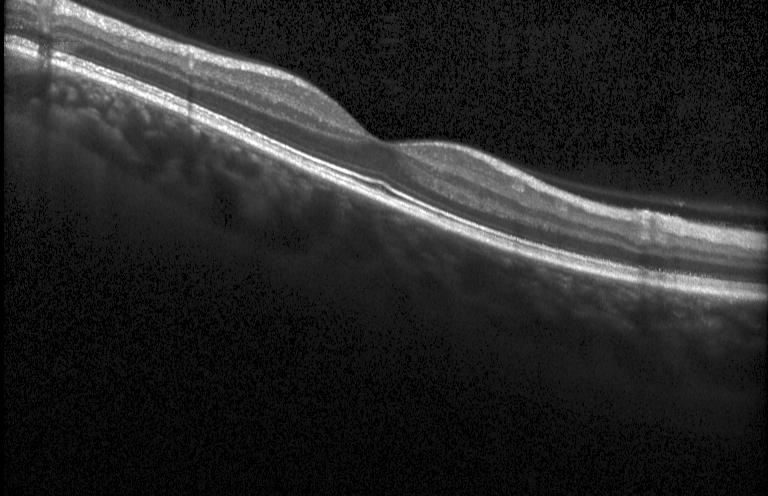

The scan shows no CNV, no DME, and no drusen.